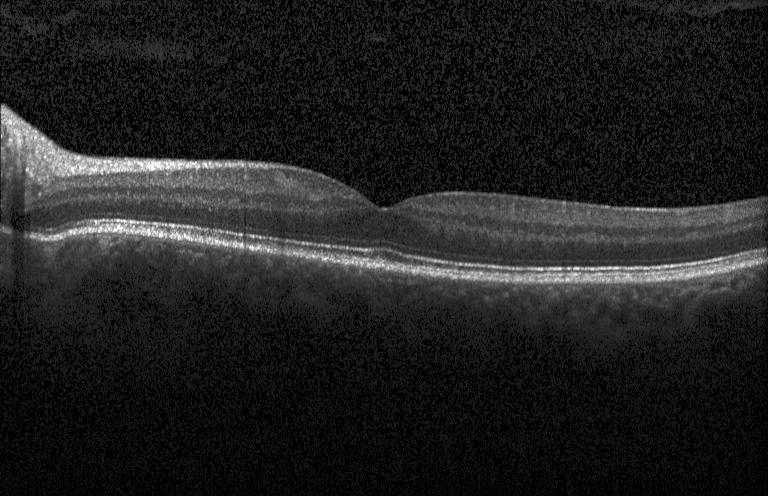 Retinal OCT cross-section showing no choroidal neovascularization, no diabetic macular edema, and no drusen.